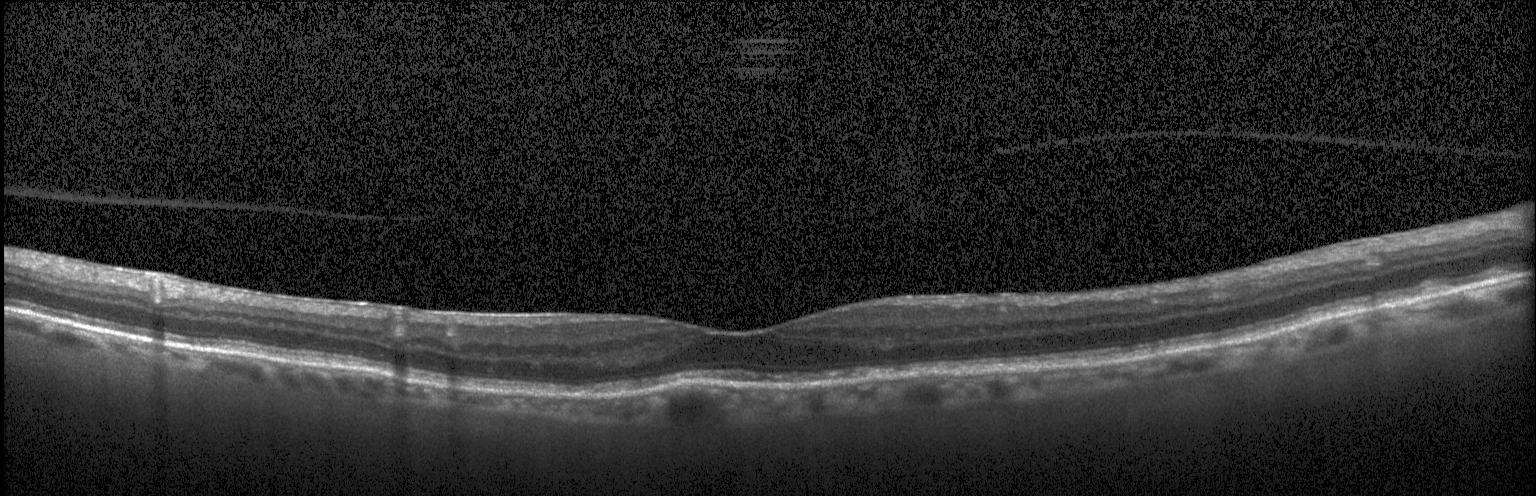
SD-OCT. Acquired on a Heidelberg Spectralis. Through the macula. OCT line scan. No evidence of CNV, DME, or drusen.